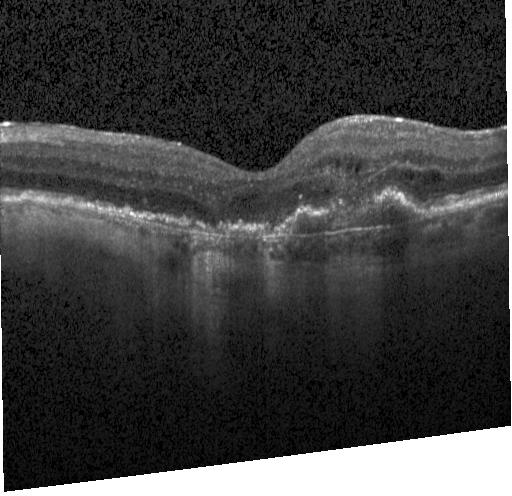 OCT B-scan showing choroidal neovascularization.